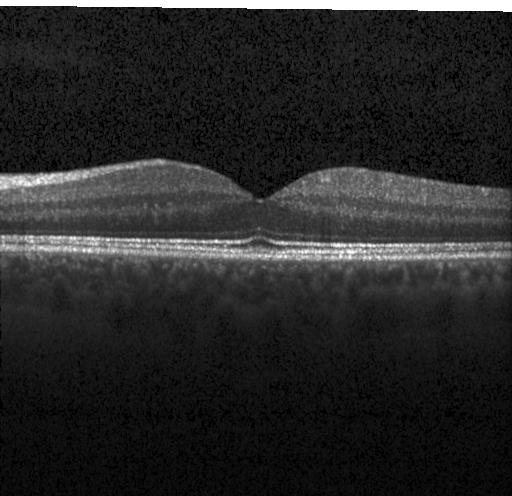 Impression: no choroidal neovascularization, no diabetic macular edema, and no drusen.